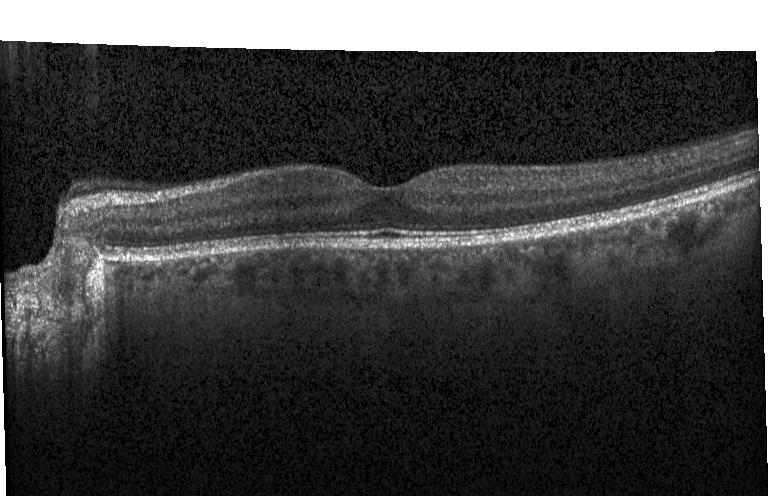 Fovea-centered · retinal OCT cross-section. This B-scan demonstrates no choroidal neovascularization, diabetic macular edema, or drusen.